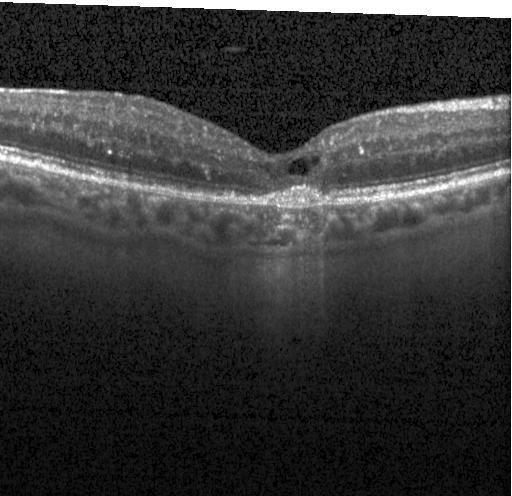
Retinal OCT cross-section.
Dx: a choroidal neovascular membrane.